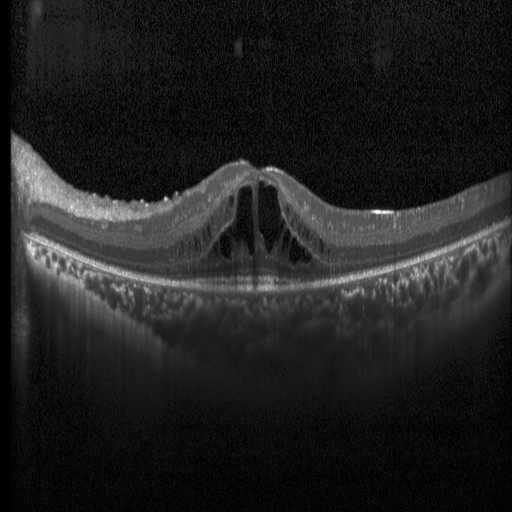
Diagnosis: diabetic macular edema (DME).